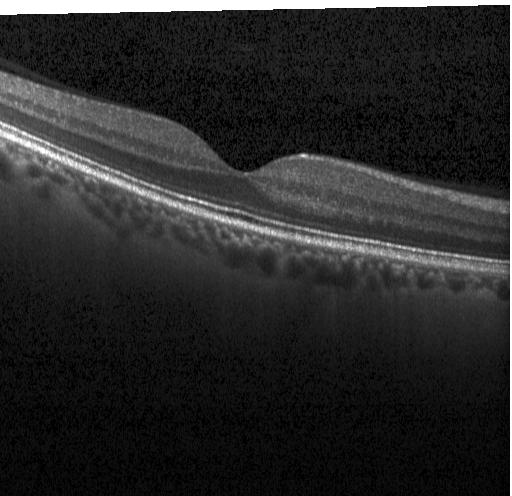

Fovea-centered; optical coherence tomography scan; SD-OCT — The scan shows neither choroidal neovascularization, diabetic macular edema, nor drusen.